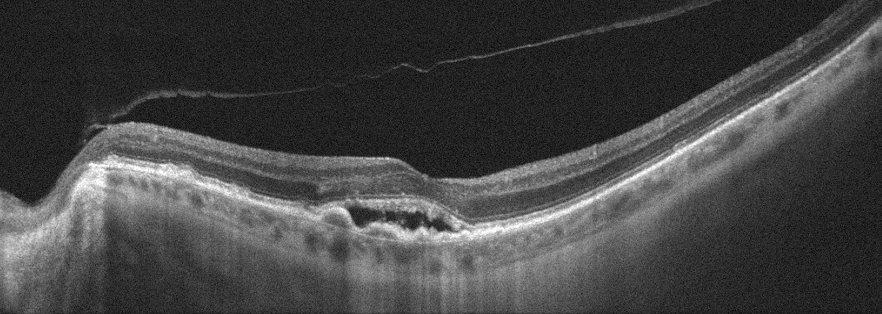 Oculus sinister, retinal OCT B-scan, acquired on an Optovue Avanti RTVue XR, through the macula. Diagnosis: age-related macular degeneration (AMD).